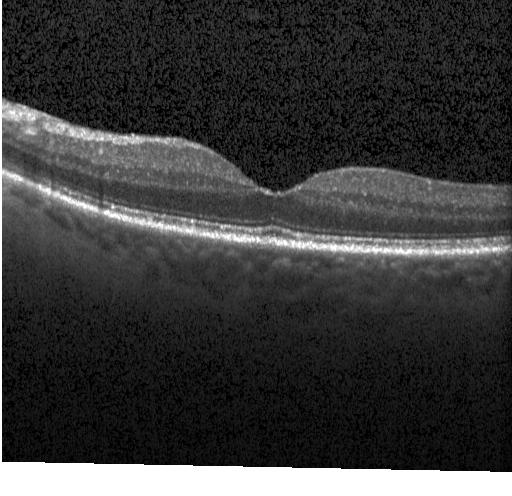

The scan shows no choroidal neovascularization, diabetic macular edema, or drusen.